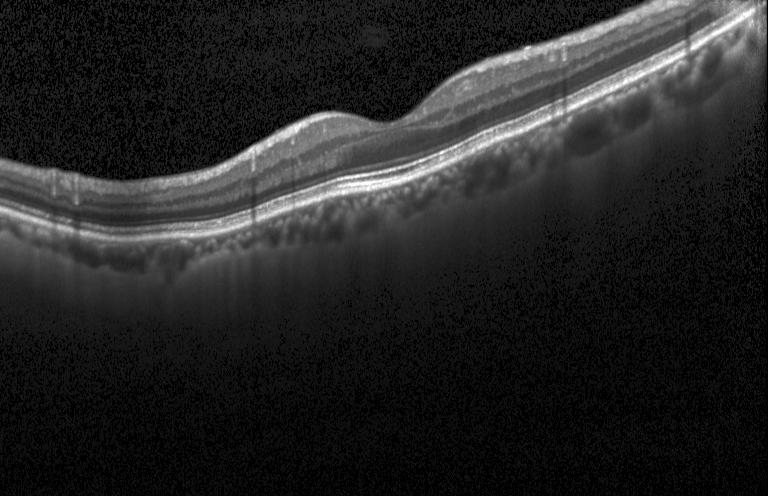

OCT B-scan. OCT finding: no CNV, DME, or drusen.